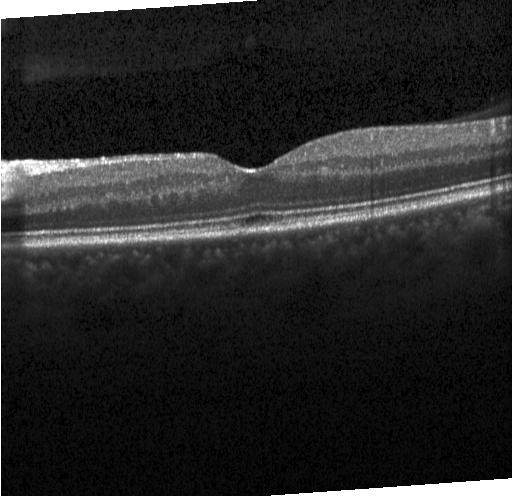
Spectral-domain optical coherence tomography · centered on the fovea · OCT line scan.
Finding: neither CNV, DME, nor drusen.